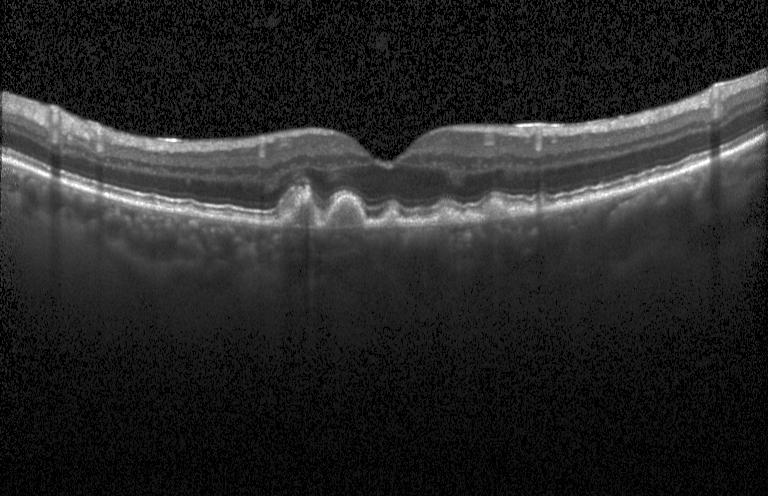

Finding: sub-RPE drusenoid deposits.